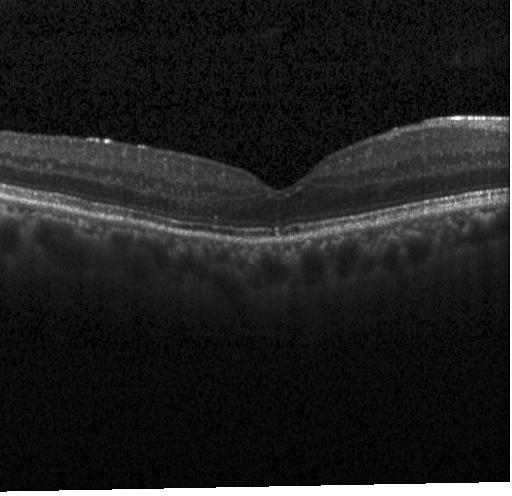 This B-scan demonstrates no choroidal neovascularization, no diabetic macular edema, and no drusen.